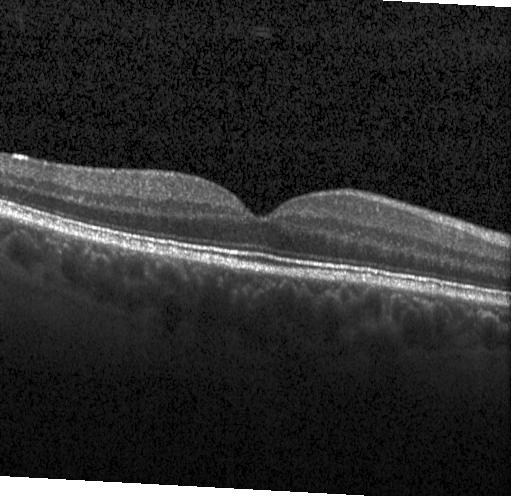 Heidelberg Spectralis · optical coherence tomography scan · centered on the fovea
This B-scan demonstrates no CNV, DME, or drusen.